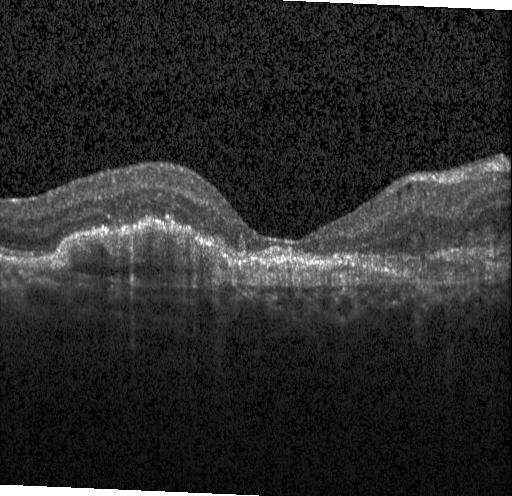
The scan shows choroidal neovascularization (CNV).